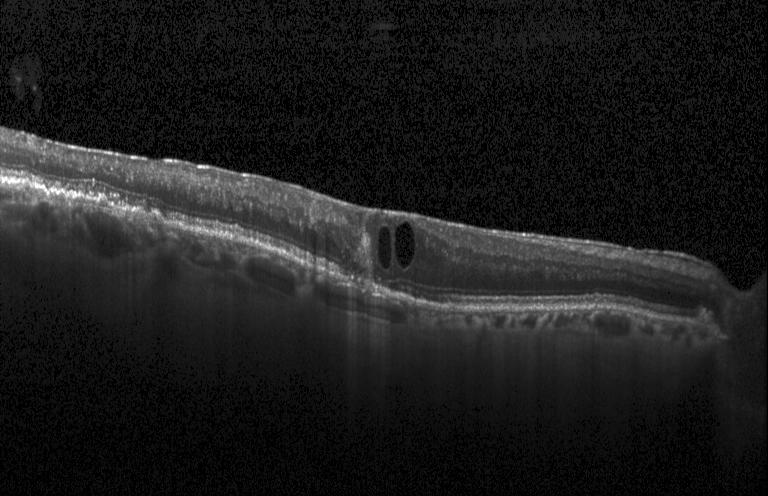

Macular OCT: choroidal neovascularization (CNV).